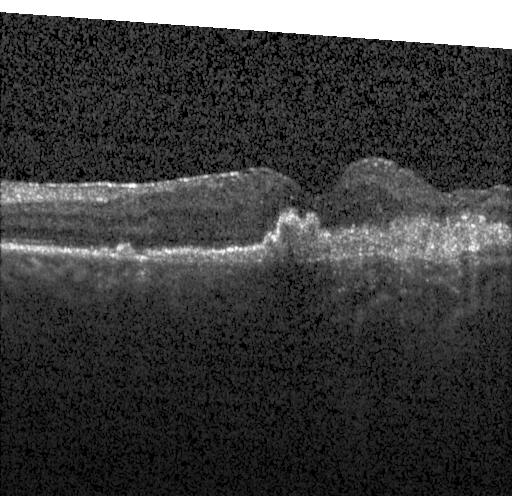

Finding: CNV.